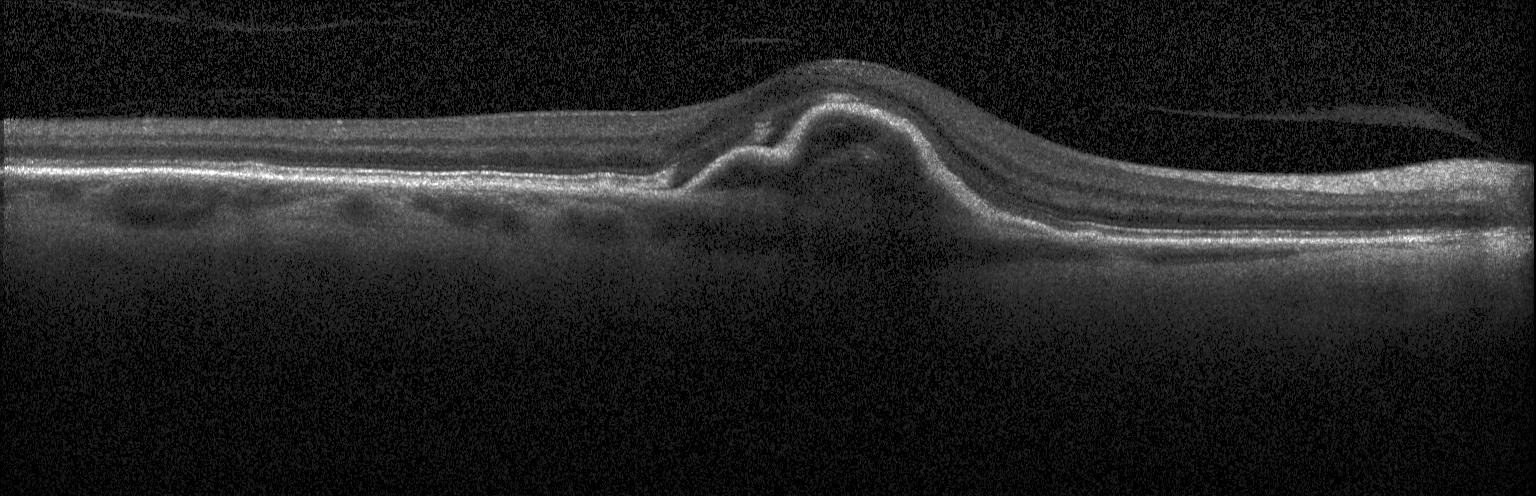

Macular scan, OCT B-scan.
OCT finding: a choroidal neovascular membrane.